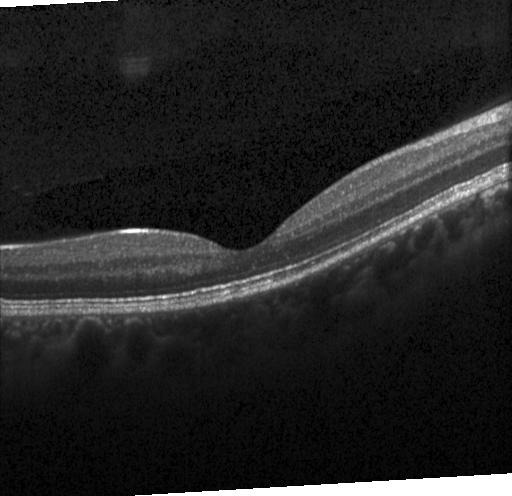

Retinal OCT B-scan — This B-scan demonstrates neither choroidal neovascularization, diabetic macular edema, nor drusen.